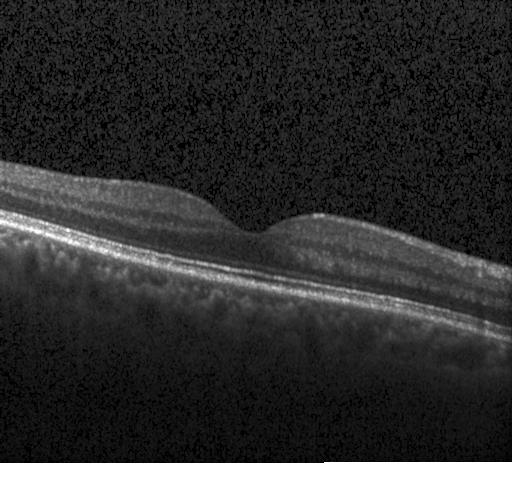 Retinal OCT cross-section, spectral-domain optical coherence tomography. The scan shows neither CNV, DME, nor drusen.